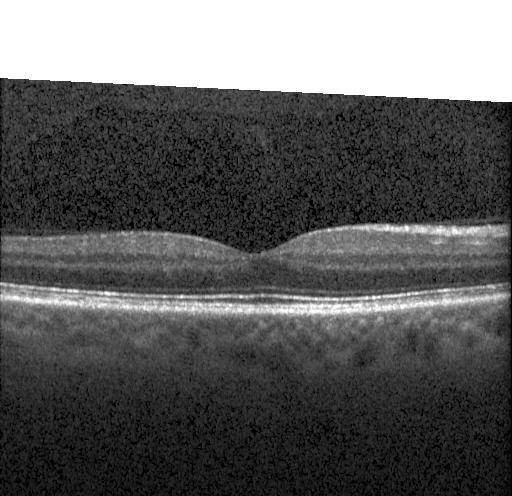
OCT line scan. Heidelberg Spectralis. Fovea-centered. Spectral-domain optical coherence tomography — Macular OCT: no choroidal neovascularization, diabetic macular edema, or drusen.